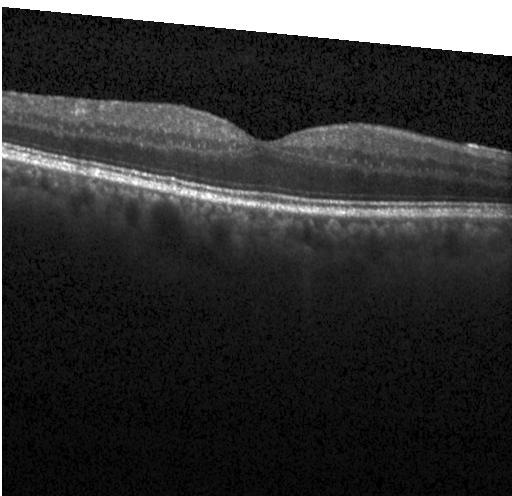
Centered on the fovea · instrument: Heidelberg Spectralis · optical coherence tomography B-scan.
The scan shows no choroidal neovascularization, diabetic macular edema, or drusen.